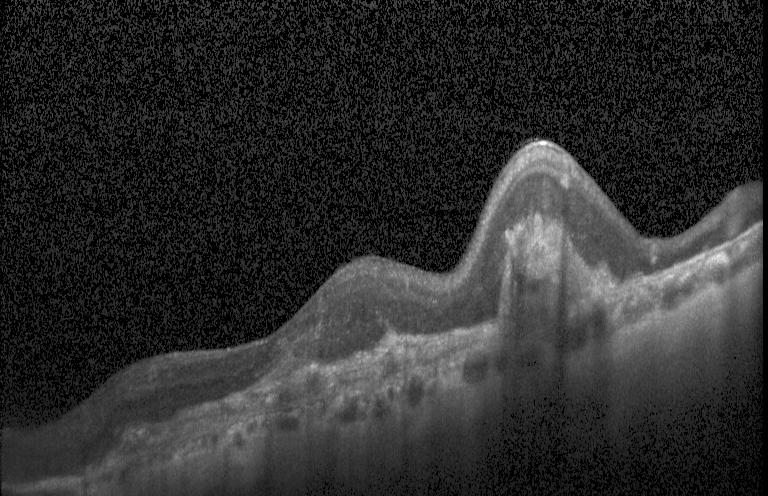
Diagnosis: choroidal neovascularization.